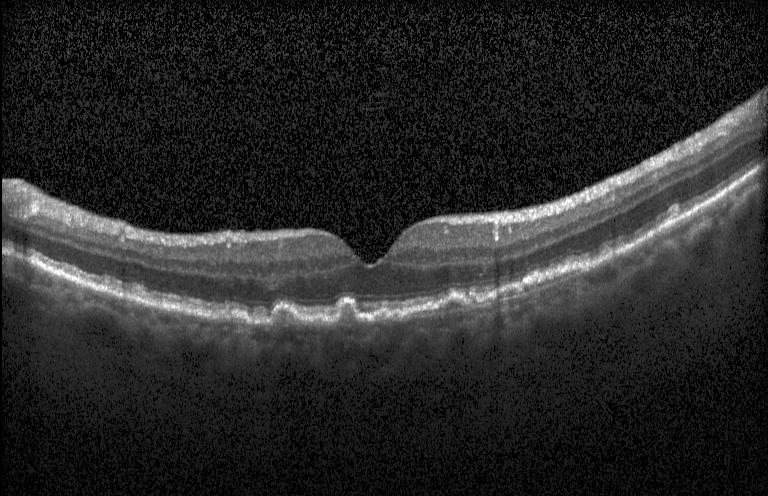
Optical coherence tomography scan · Heidelberg Spectralis OCT system.
Assessment: sub-RPE drusenoid deposits.